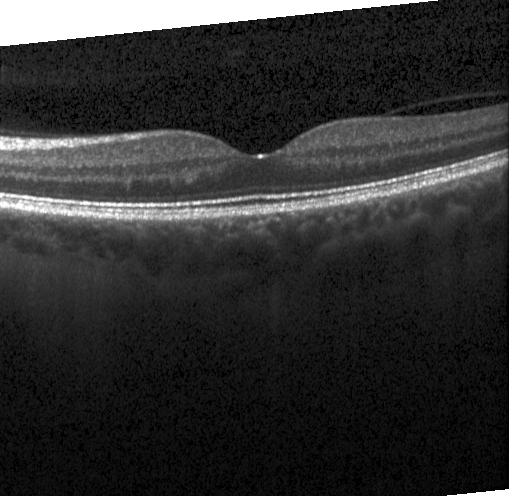
Fovea-centered. Heidelberg Spectralis. OCT line scan. SD-OCT
The scan shows no choroidal neovascularization, no diabetic macular edema, and no drusen.